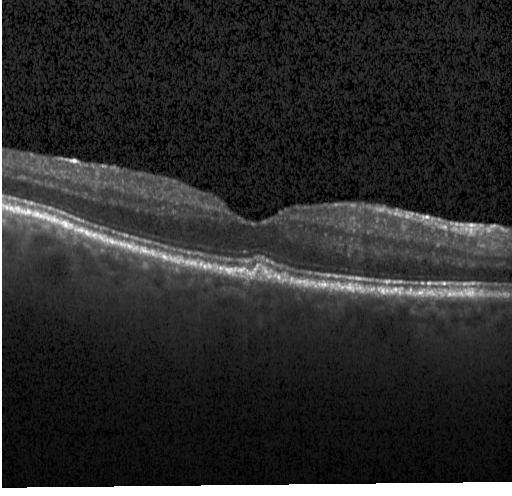
OCT B-scan, spectral-domain optical coherence tomography. OCT finding: sub-RPE drusenoid deposits.